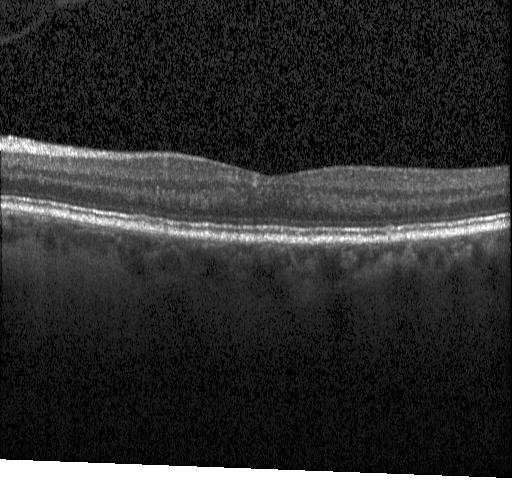

Finding: no choroidal neovascularization, no diabetic macular edema, and no drusen.